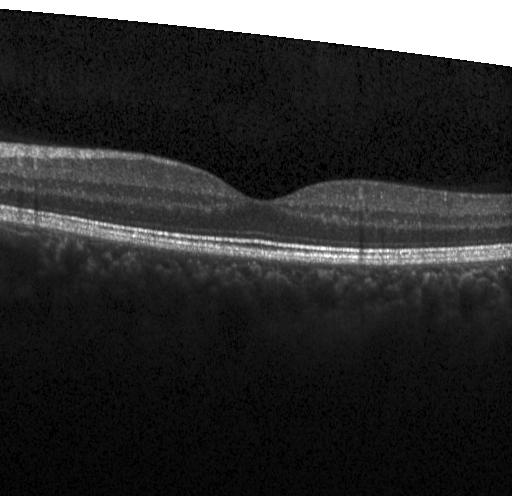

Spectral-domain optical coherence tomography · fovea-centered · acquired on a Heidelberg Spectralis · retinal OCT cross-section
Impression: no evidence of choroidal neovascularization, diabetic macular edema, or drusen.